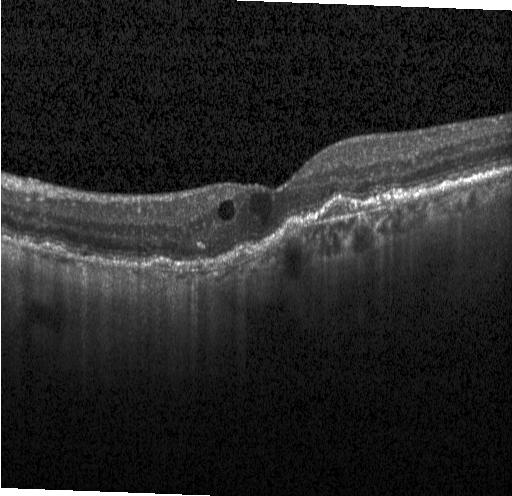 SD-OCT; acquired on a Heidelberg Spectralis; retinal OCT cross-section.
The scan shows choroidal neovascularization (CNV).